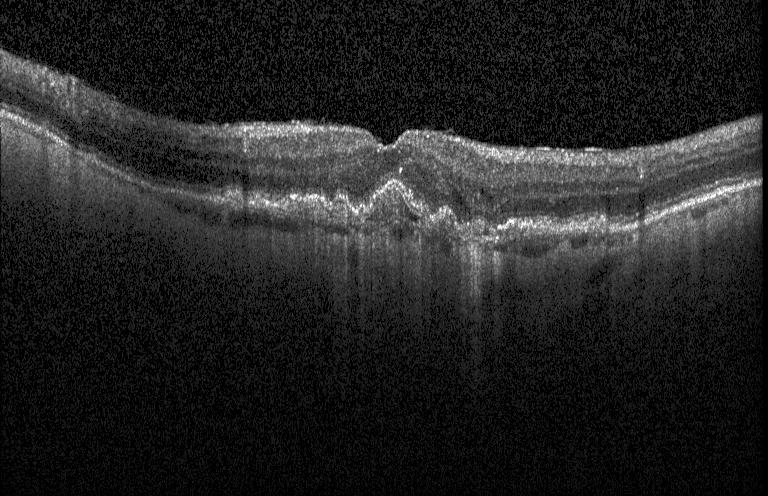 Heidelberg Spectralis OCT system; horizontal scan through the fovea; SD-OCT; optical coherence tomography B-scan.
This B-scan demonstrates a choroidal neovascular membrane.